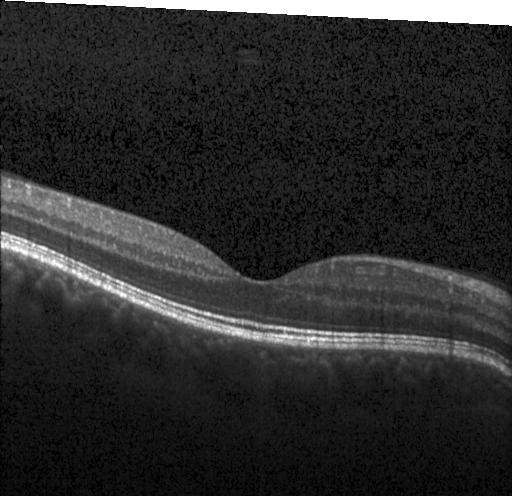 OCT B-scan.
Finding: no evidence of CNV, DME, or drusen.